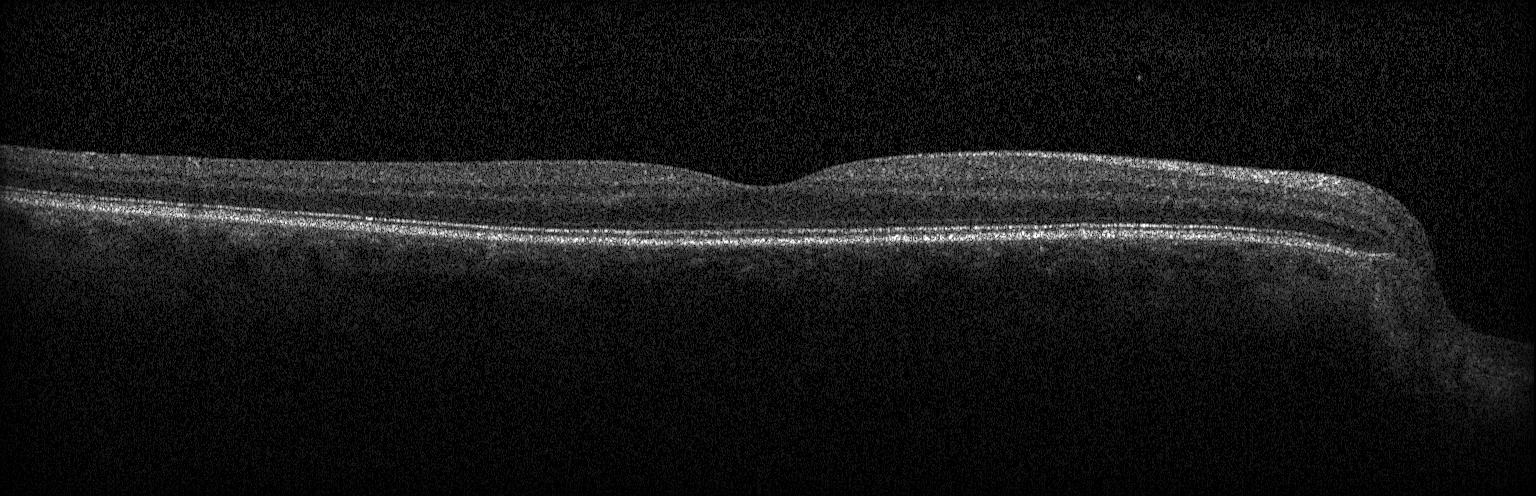

Optical coherence tomography B-scan. Fovea-centered. Spectral-domain OCT
The scan shows no evidence of choroidal neovascularization, diabetic macular edema, or drusen.